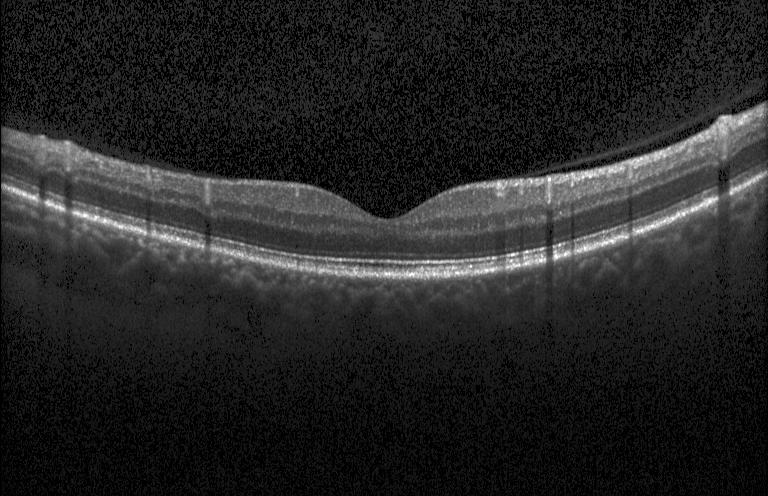 Dx: no choroidal neovascularization, diabetic macular edema, or drusen.